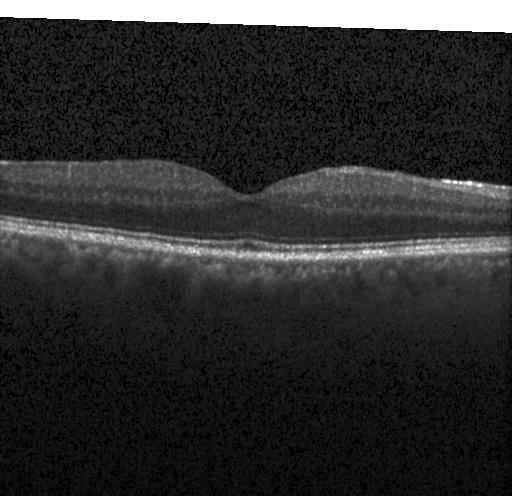

Finding: no choroidal neovascularization, diabetic macular edema, or drusen.